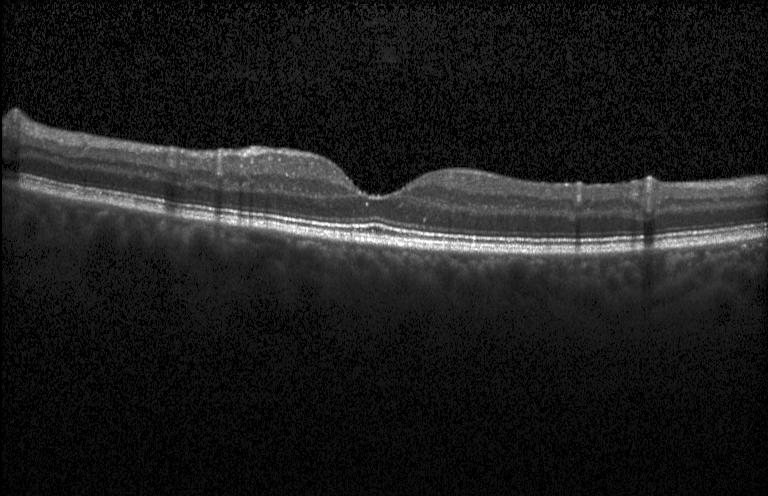 OCT line scan, fovea-centered, Heidelberg Spectralis OCT system, SD-OCT
Diagnosis: no choroidal neovascularization, diabetic macular edema, or drusen.